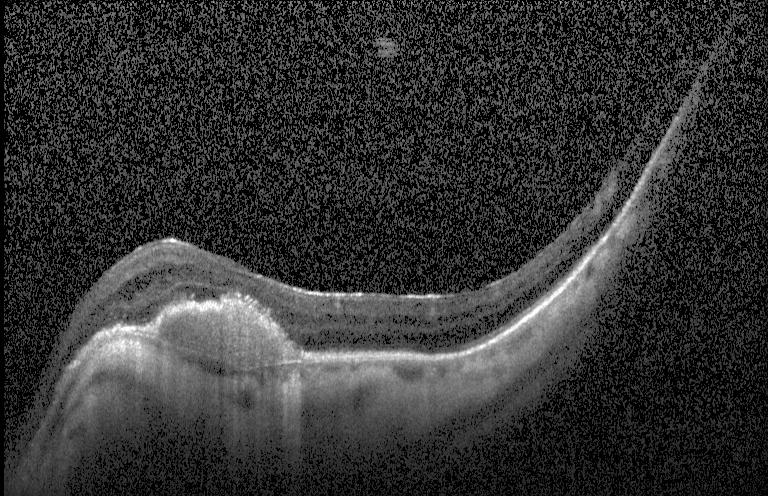

OCT B-scan — Diagnosis: choroidal neovascularization.